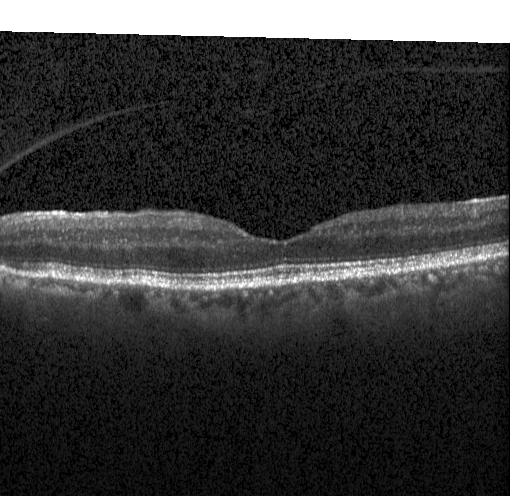

Dx: neither CNV, DME, nor drusen.